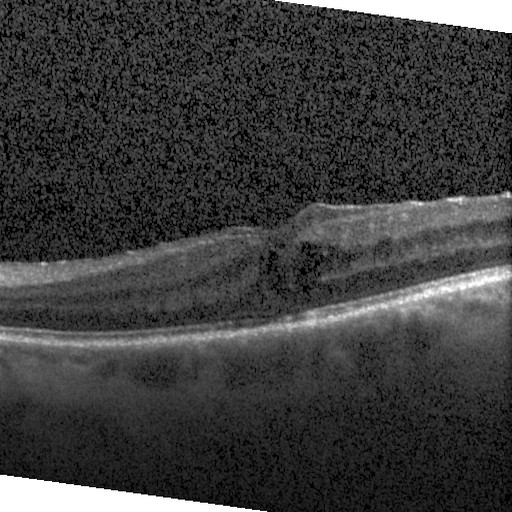

Heidelberg Spectralis OCT system · through the macula · OCT line scan — Macular OCT: diabetic macular edema.